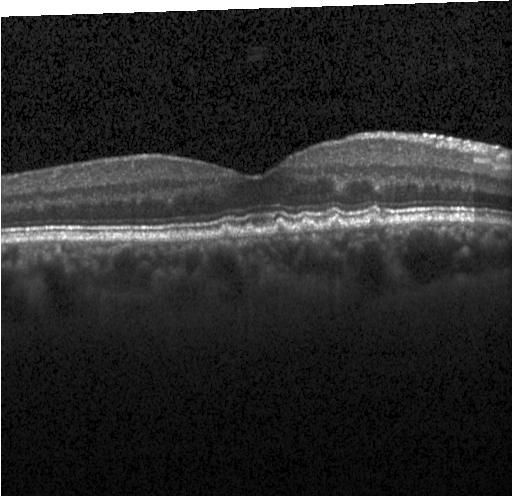

OCT B-scan showing drusen.